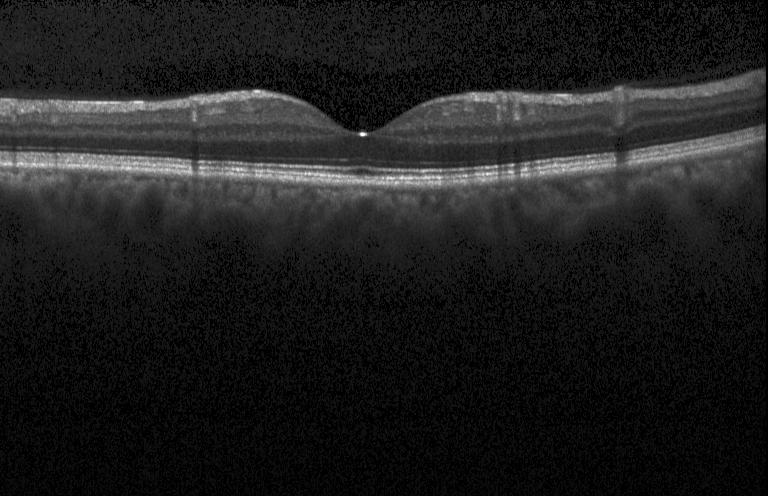

Diagnosis: neither CNV, DME, nor drusen.